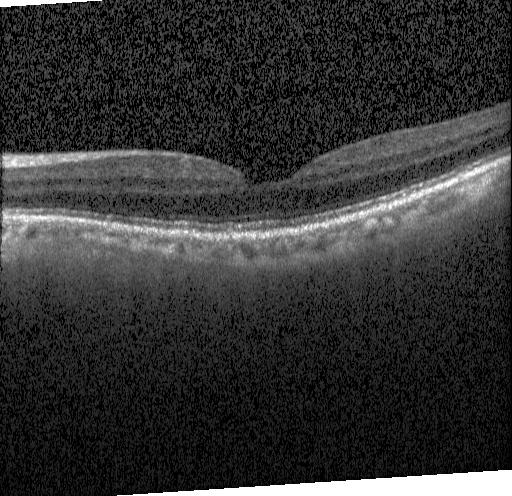
OCT line scan, Heidelberg Spectralis OCT system, spectral-domain OCT, horizontal scan through the fovea. The scan shows no choroidal neovascularization, no diabetic macular edema, and no drusen.